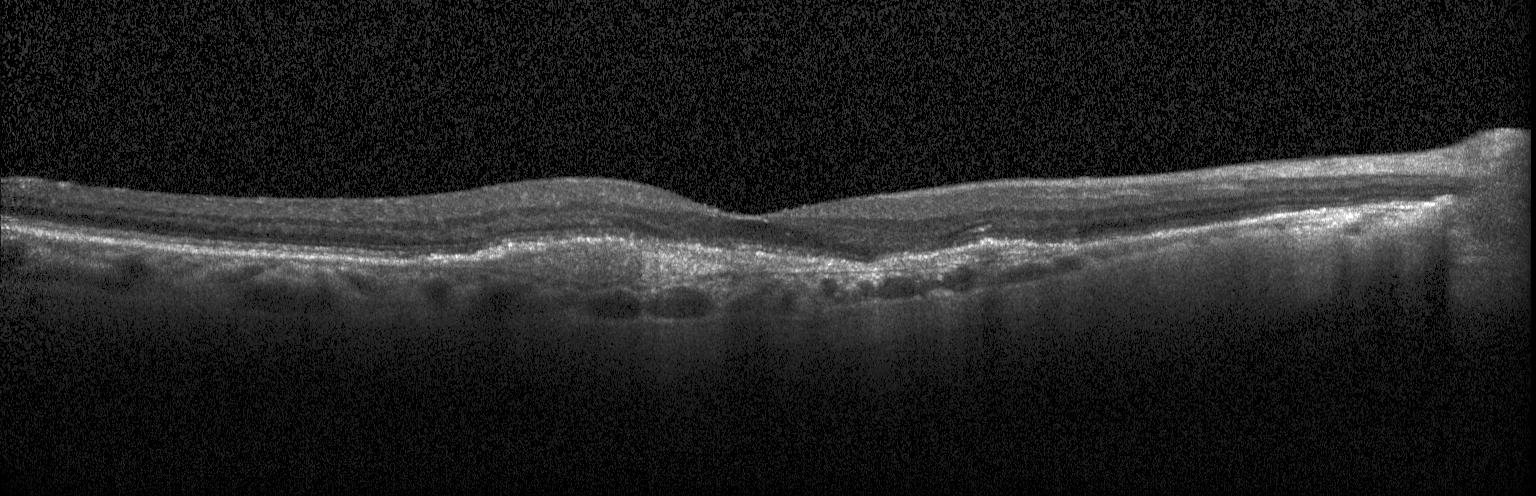
Spectral-domain optical coherence tomography; retinal OCT B-scan; instrument: Heidelberg Spectralis.
This B-scan demonstrates a choroidal neovascular membrane.